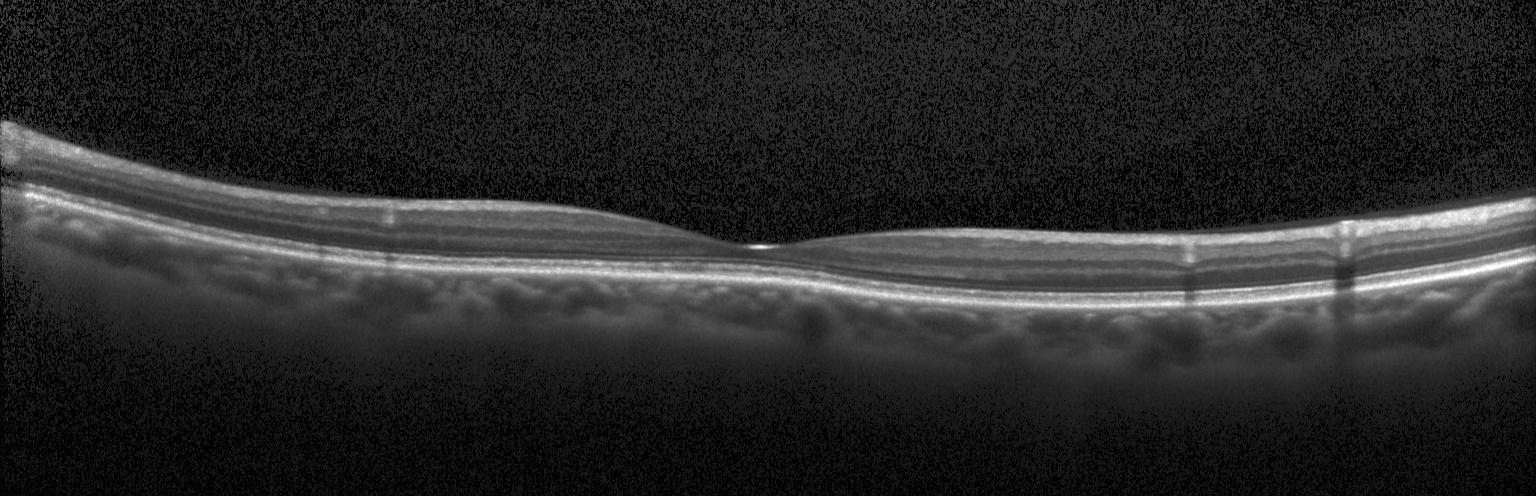 Optical coherence tomography B-scan · fovea-centered · spectral-domain optical coherence tomography · instrument: Heidelberg Spectralis.
The scan shows no choroidal neovascularization, diabetic macular edema, or drusen.